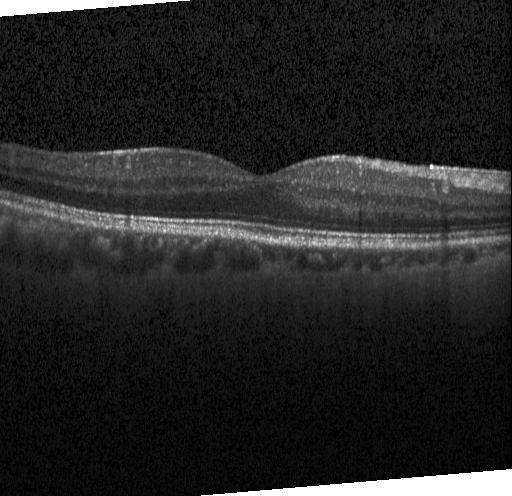
Impression: no CNV, DME, or drusen.